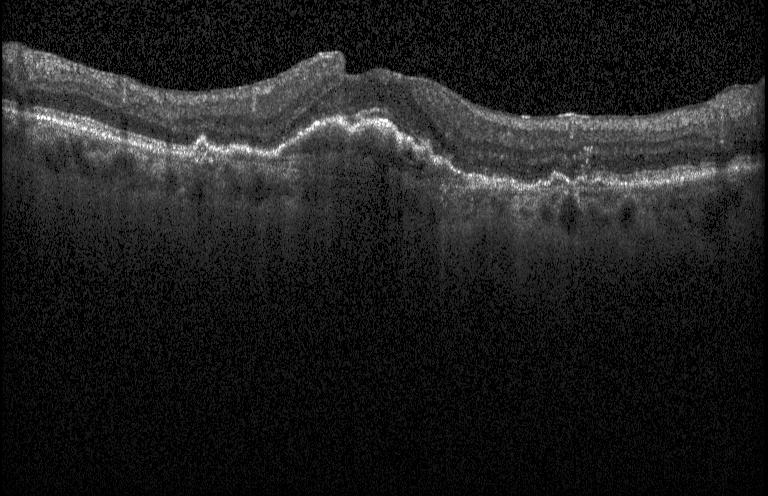

OCT line scan
Finding: choroidal neovascularization.